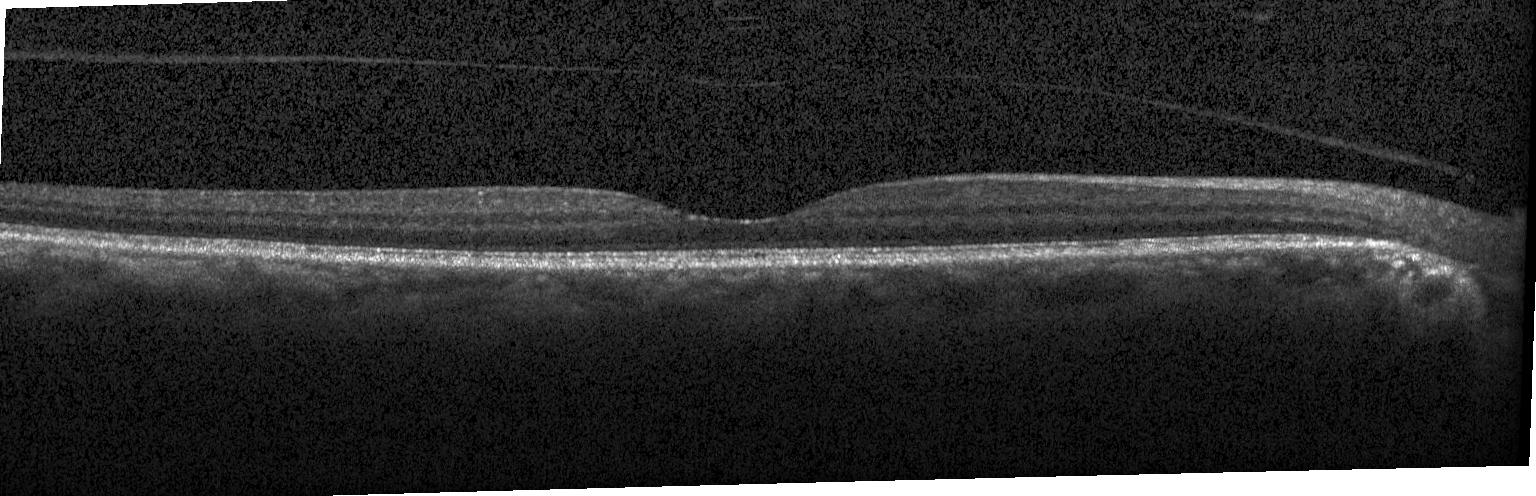
Spectral-domain optical coherence tomography; acquired on a Heidelberg Spectralis; retinal OCT cross-section.
Impression: no CNV, no DME, and no drusen.